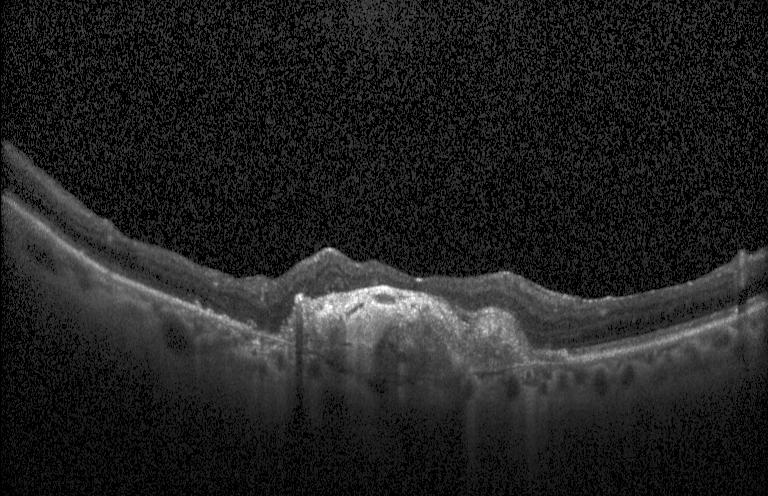

Instrument: Heidelberg Spectralis · OCT line scan — Macular OCT: a choroidal neovascular membrane.